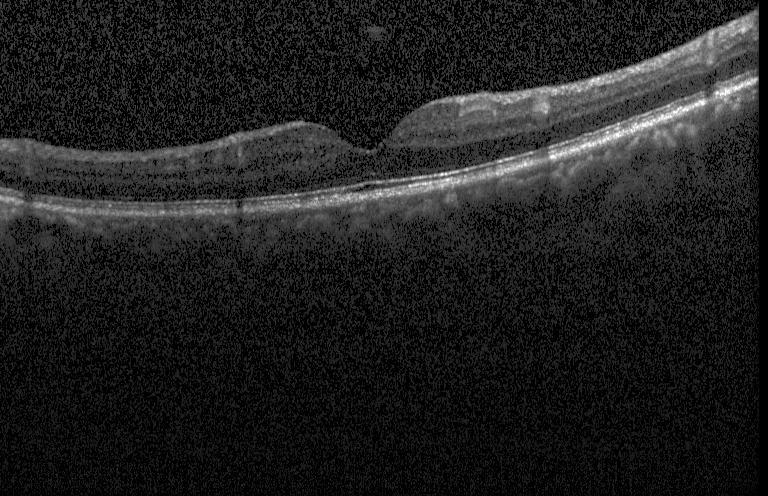 Macular OCT: no evidence of CNV, DME, or drusen.